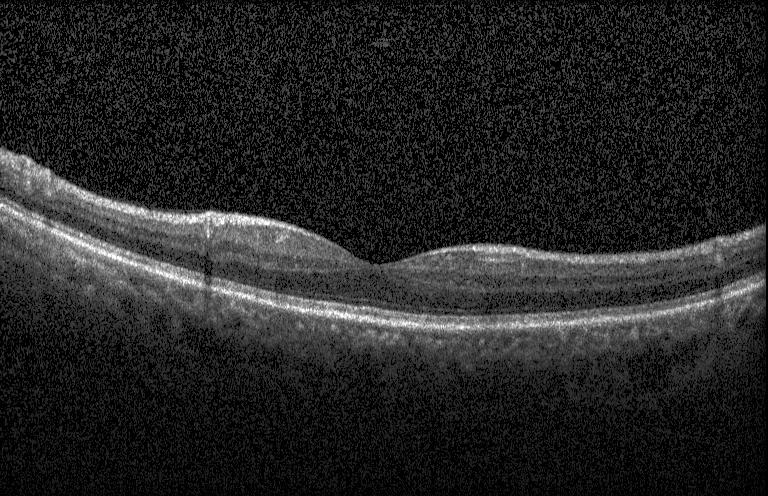
Optical coherence tomography B-scan. SD-OCT. Heidelberg Spectralis.
Dx: neither choroidal neovascularization, diabetic macular edema, nor drusen.